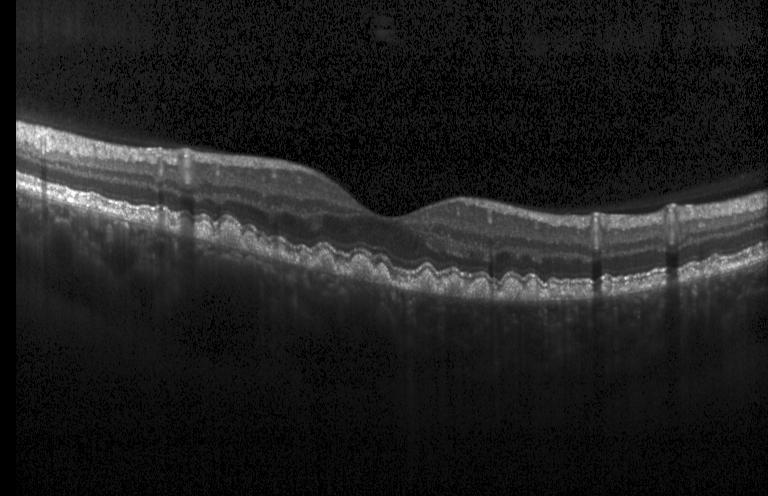

Sub-RPE drusenoid deposits.